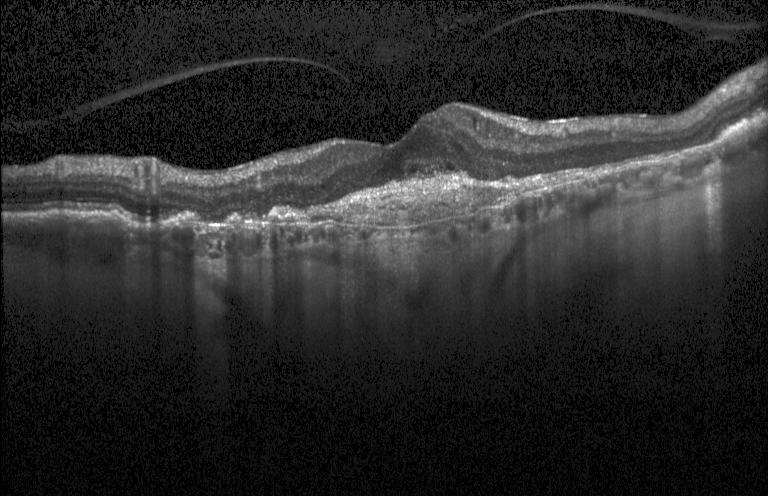 Acquired on a Heidelberg Spectralis · centered on the fovea · OCT line scan — Choroidal neovascularization (CNV).